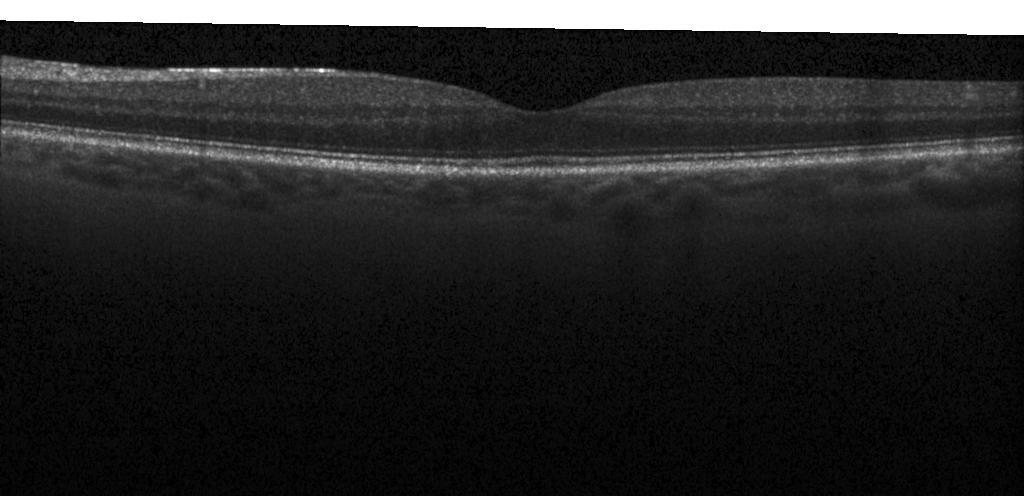

Retinal OCT cross-section showing no evidence of choroidal neovascularization, diabetic macular edema, or drusen.